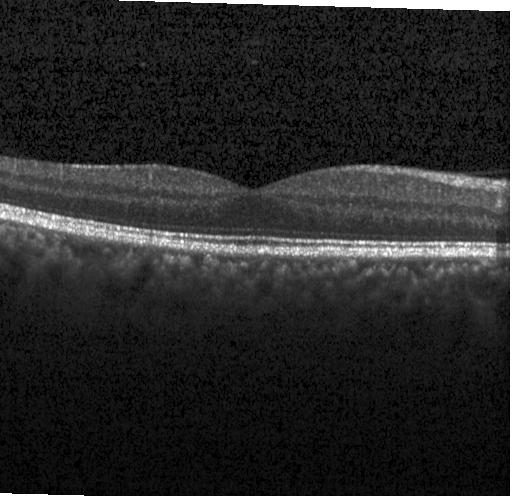 Instrument: Heidelberg Spectralis; spectral-domain OCT; optical coherence tomography B-scan; horizontal scan through the fovea.
Assessment: no evidence of CNV, DME, or drusen.